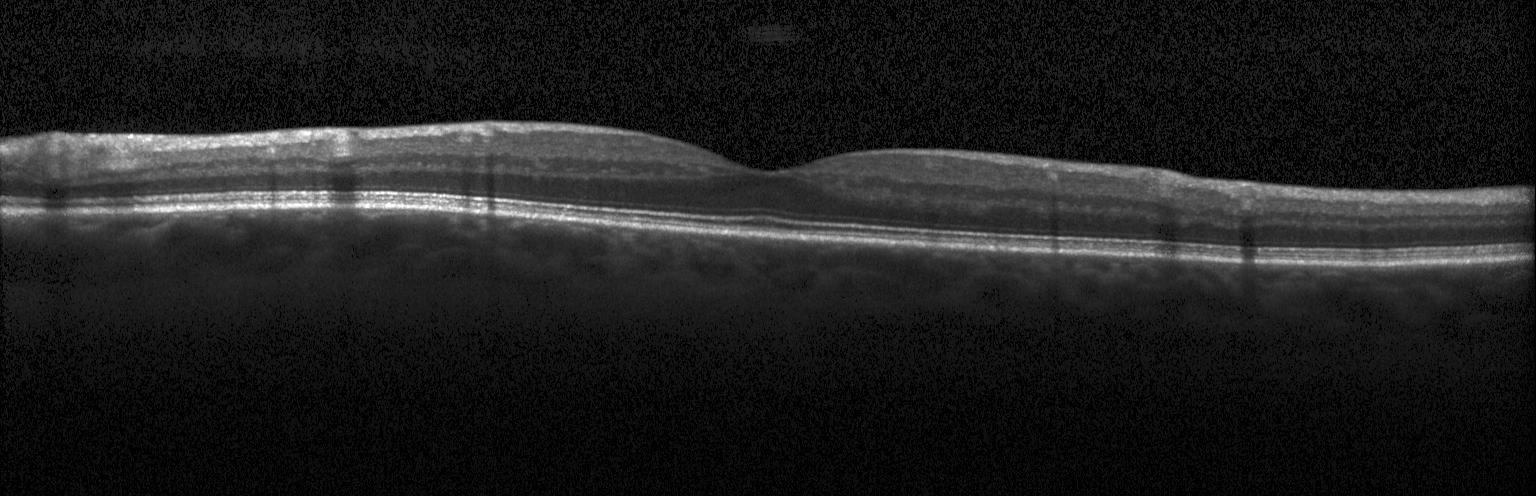
SD-OCT · retinal OCT B-scan
Impression: no choroidal neovascularization, no diabetic macular edema, and no drusen.